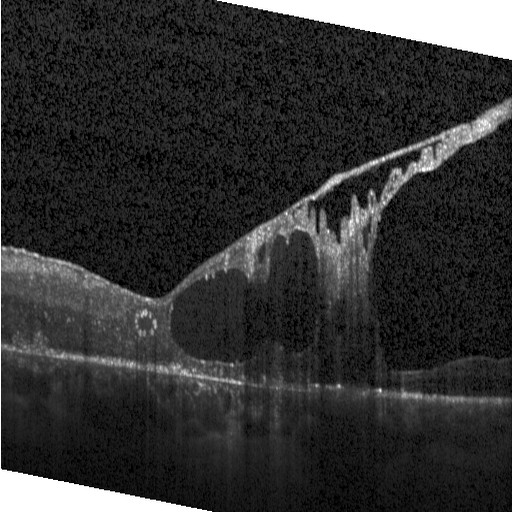 Optical coherence tomography scan — The scan shows diabetic macular edema (DME).